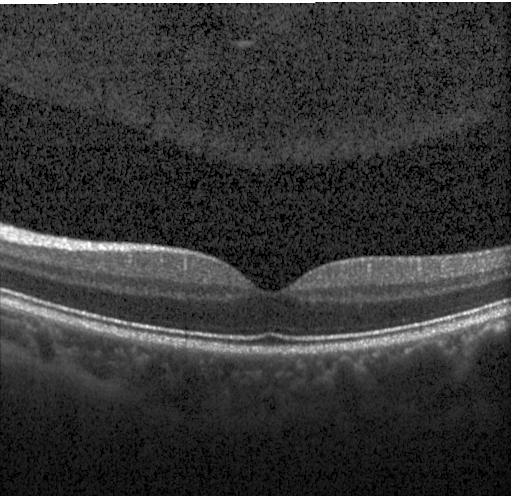
Impression: neither choroidal neovascularization, diabetic macular edema, nor drusen.